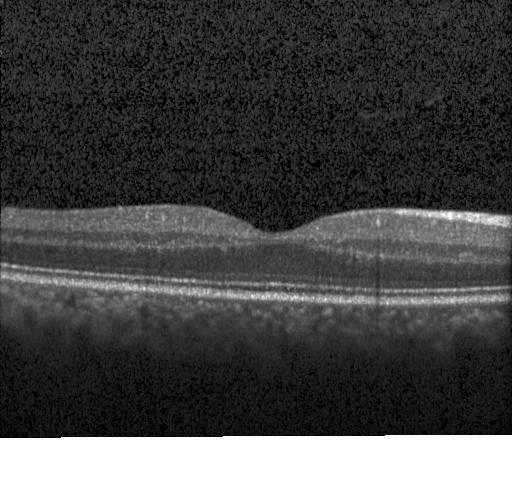

Optical coherence tomography scan — The scan shows no choroidal neovascularization, diabetic macular edema, or drusen.